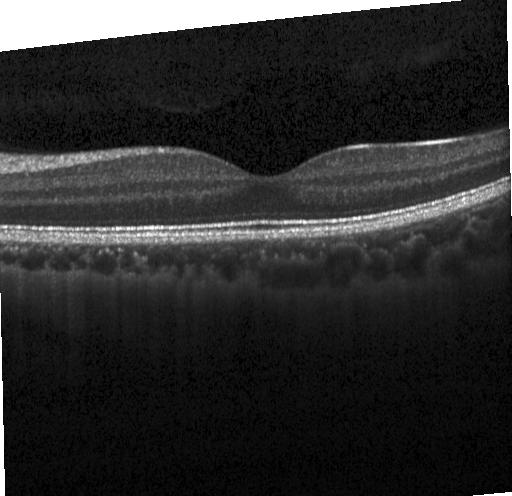 Retinal OCT B-scan. Heidelberg Spectralis. Spectral-domain optical coherence tomography.
Impression: no choroidal neovascularization, diabetic macular edema, or drusen.